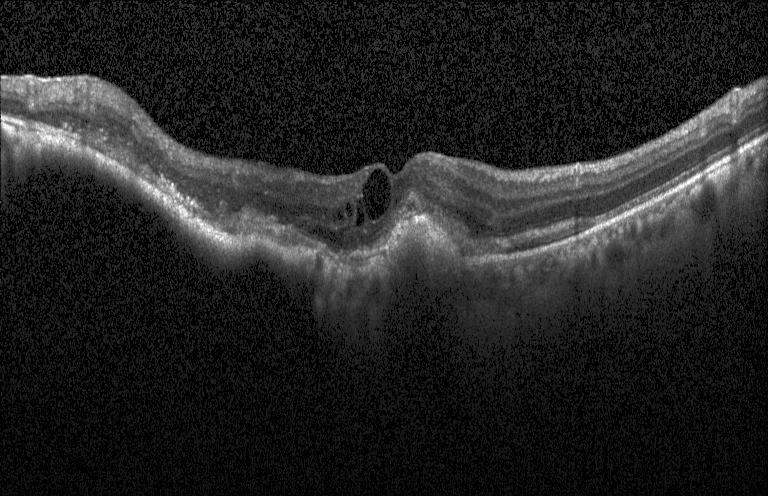 Spectral-domain optical coherence tomography. OCT line scan.
Finding: CNV.